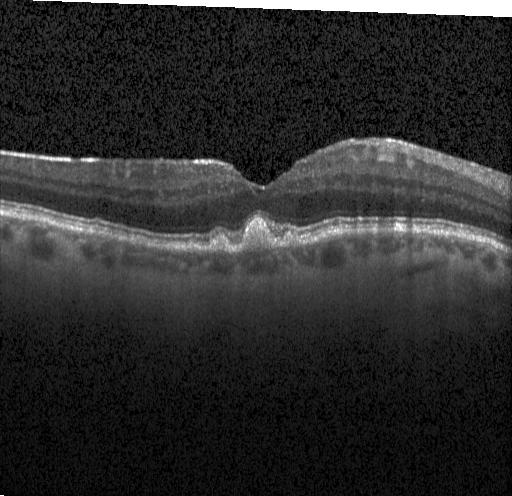
Macular OCT: multiple drusen.